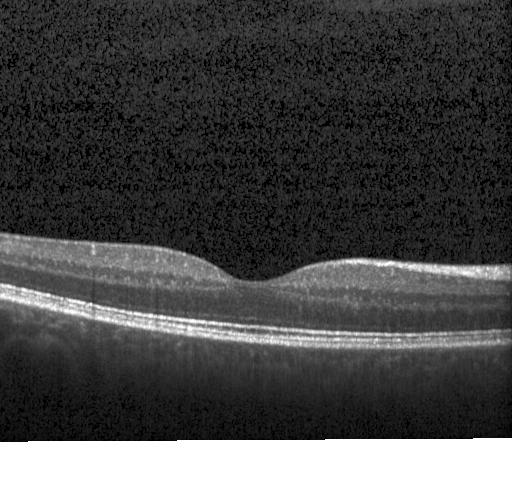 Retinal OCT B-scan
The scan shows neither CNV, DME, nor drusen.